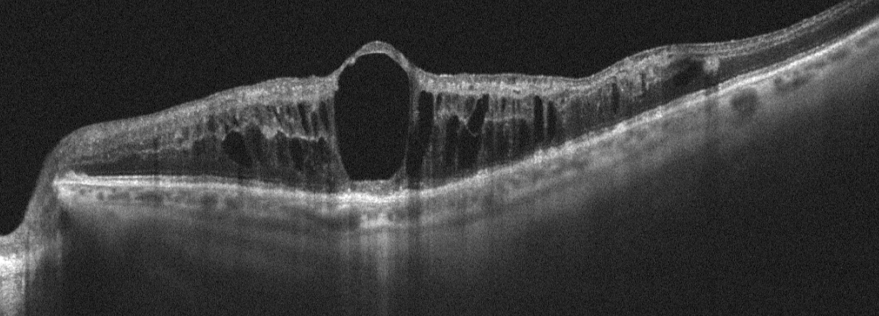 Finding: DME.